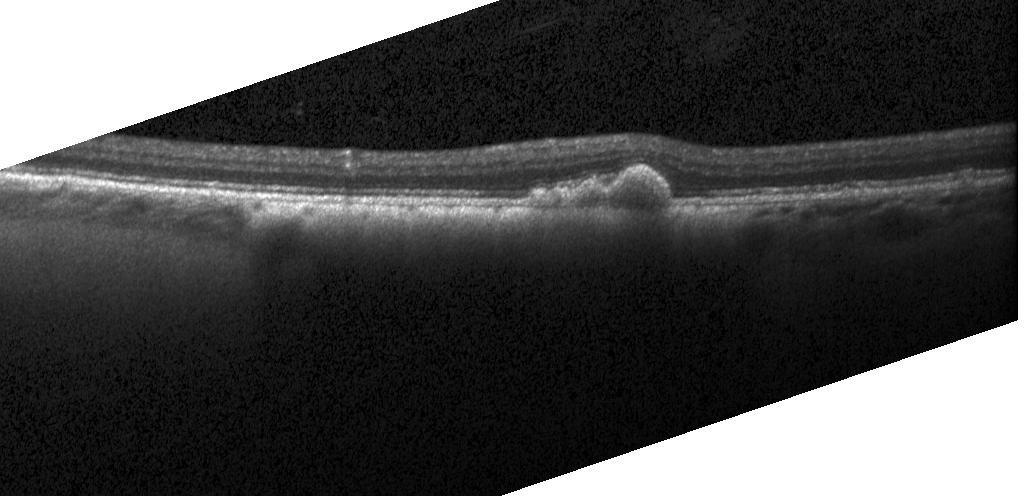 Finding: a choroidal neovascular membrane.